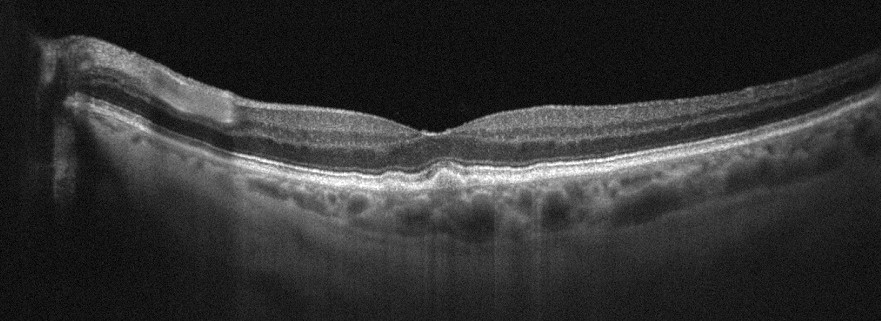

OCT finding: AMD.